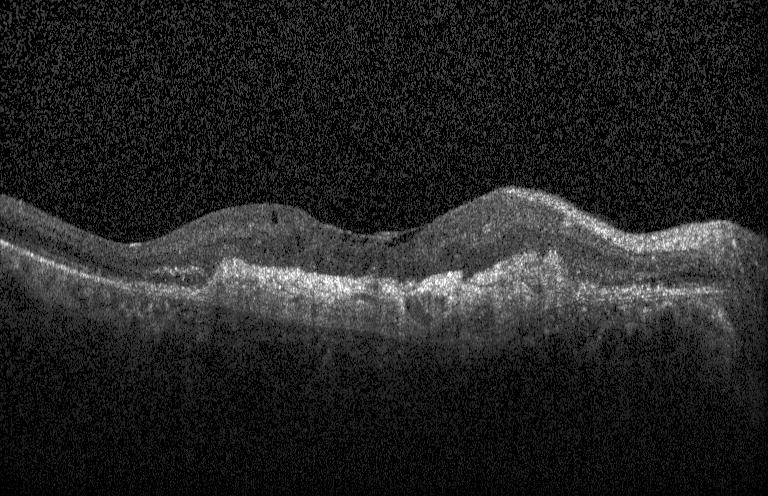

Acquired on a Heidelberg Spectralis · spectral-domain optical coherence tomography · macular scan · retinal OCT cross-section
A choroidal neovascular membrane.